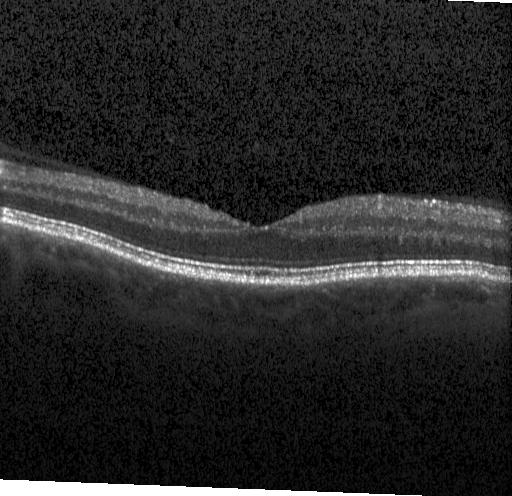

OCT finding: no choroidal neovascularization, no diabetic macular edema, and no drusen.